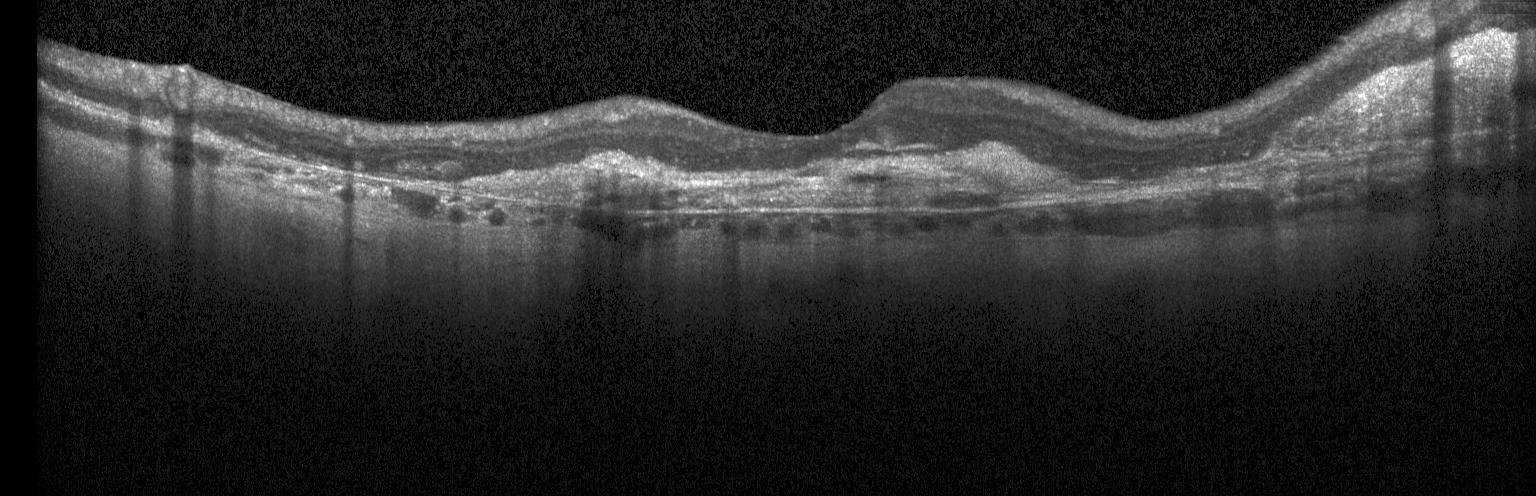
Finding: choroidal neovascularization (CNV).